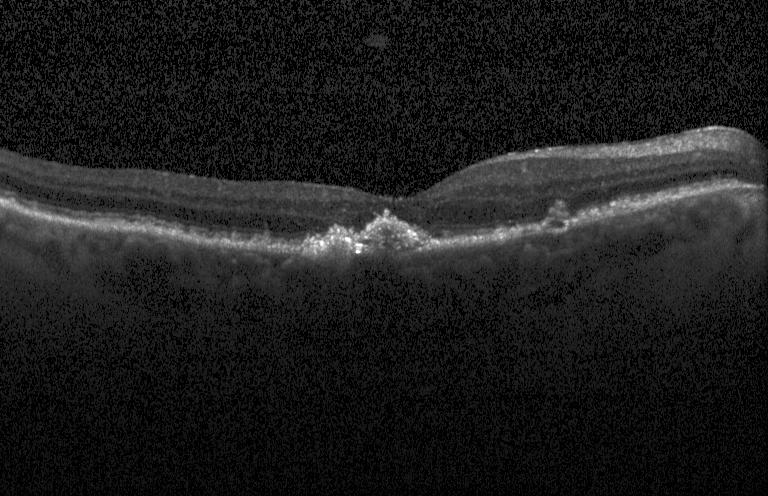 Macular OCT demonstrating CNV.